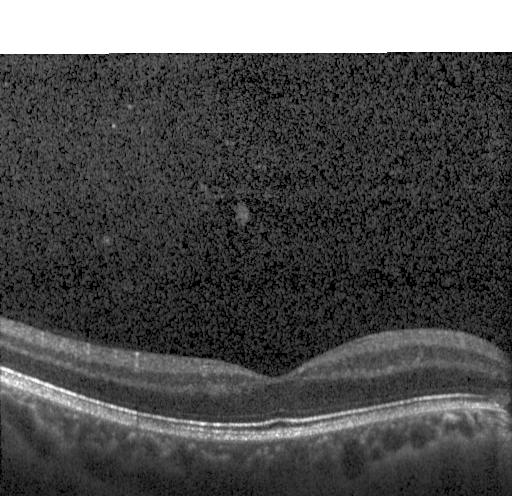
Finding: no choroidal neovascularization, no diabetic macular edema, and no drusen.